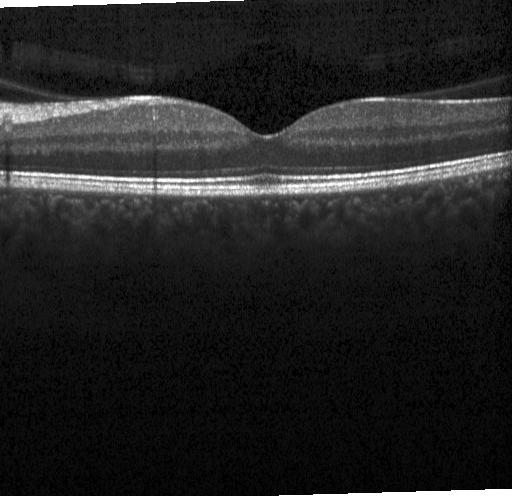

Impression: neither CNV, DME, nor drusen.